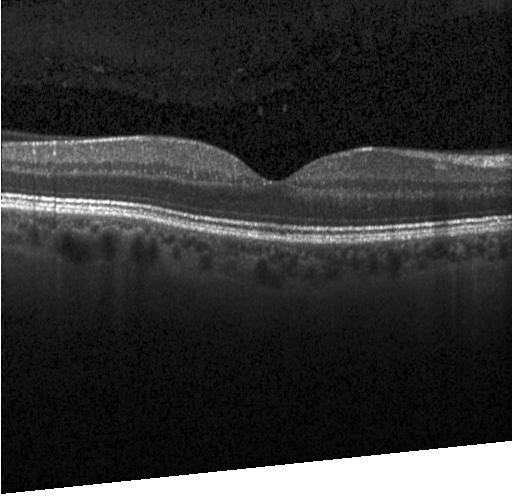

Retinal OCT cross-section; instrument: Heidelberg Spectralis; spectral-domain optical coherence tomography; horizontal scan through the fovea. This B-scan demonstrates neither choroidal neovascularization, diabetic macular edema, nor drusen.